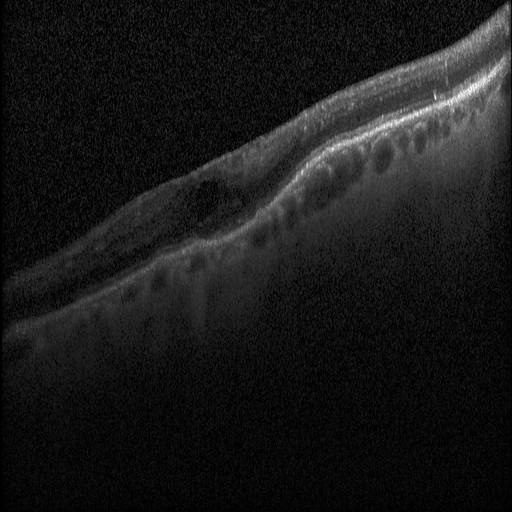

Retinal OCT B-scan. This B-scan demonstrates diabetic macular edema.